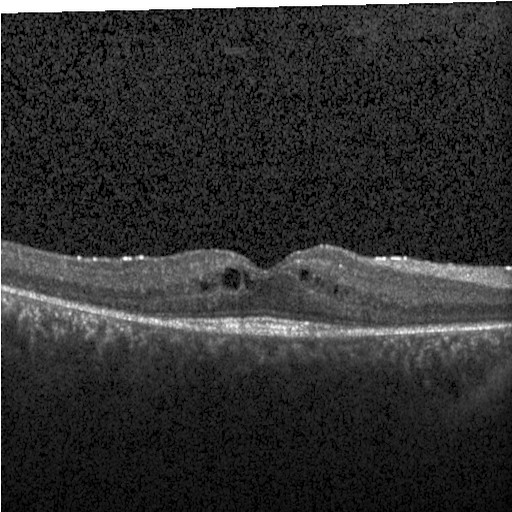
Impression: DME.